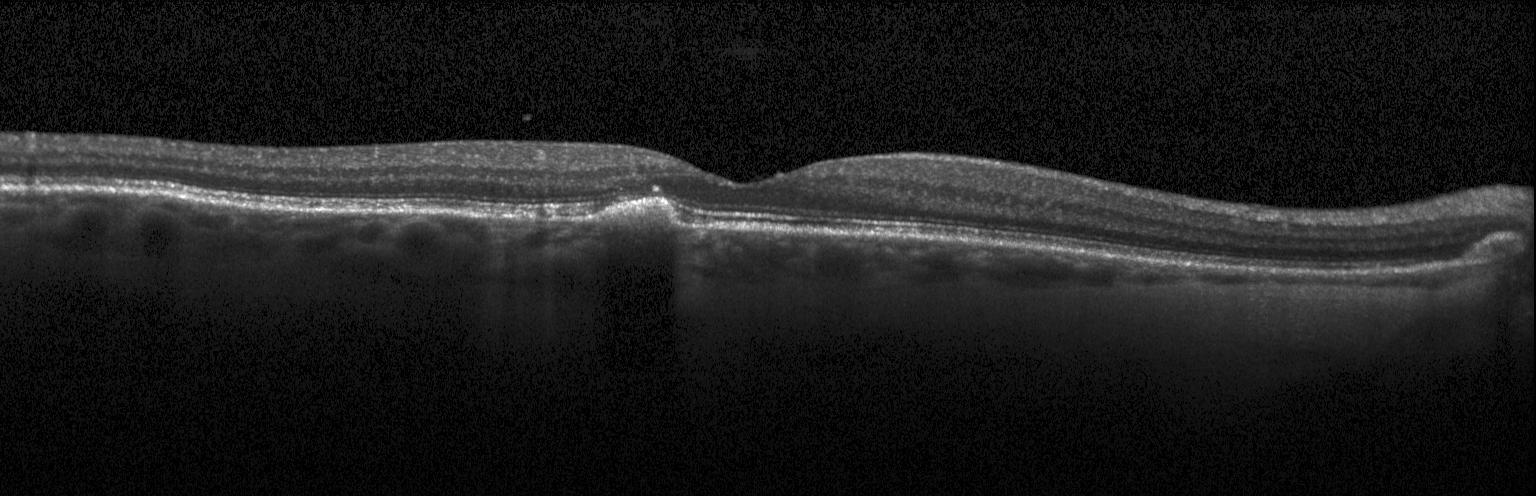

Spectral-domain OCT. Retinal OCT B-scan. Centered on the fovea. Heidelberg Spectralis
Impression: multiple drusen.